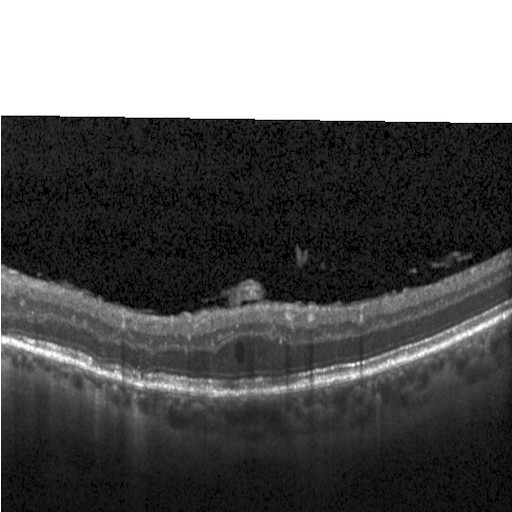
SD-OCT; horizontal scan through the fovea; OCT B-scan; instrument: Heidelberg Spectralis — Diagnosis: diabetic macular edema (DME).